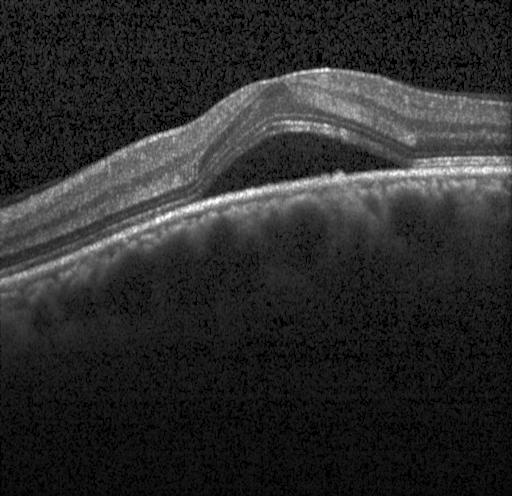 OCT finding: choroidal neovascularization.